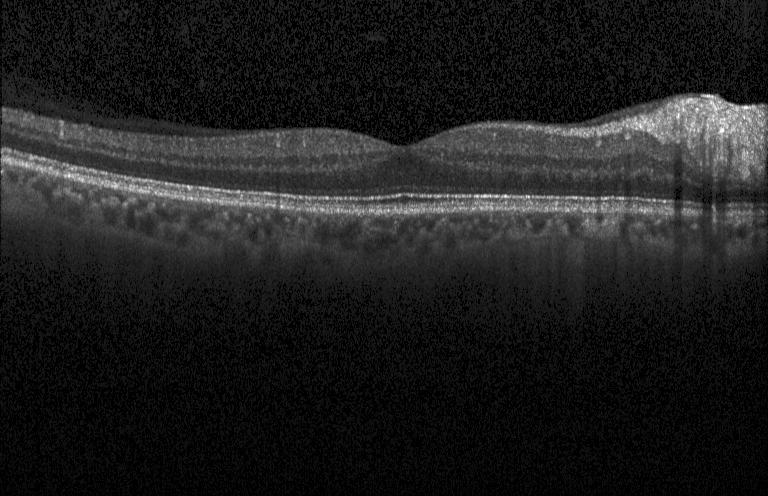 Spectral-domain OCT B-scan: no evidence of CNV, DME, or drusen.